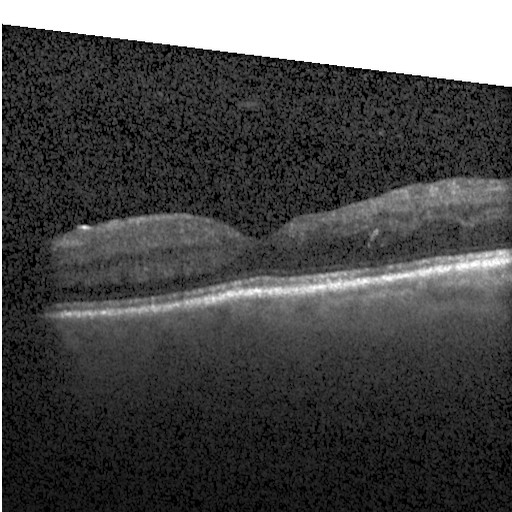 Optical coherence tomography B-scan — Macular OCT: diabetic macular edema.